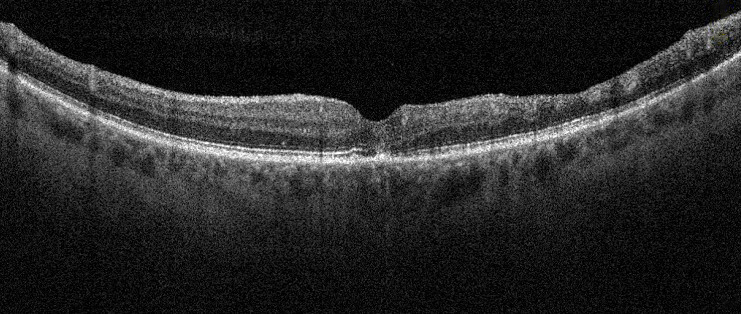 Finding: retinal vein occlusion.